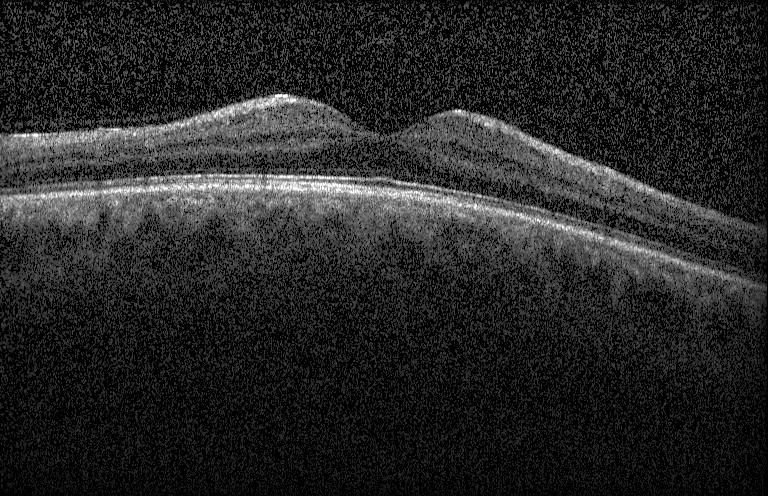
Diagnosis: neither choroidal neovascularization, diabetic macular edema, nor drusen.